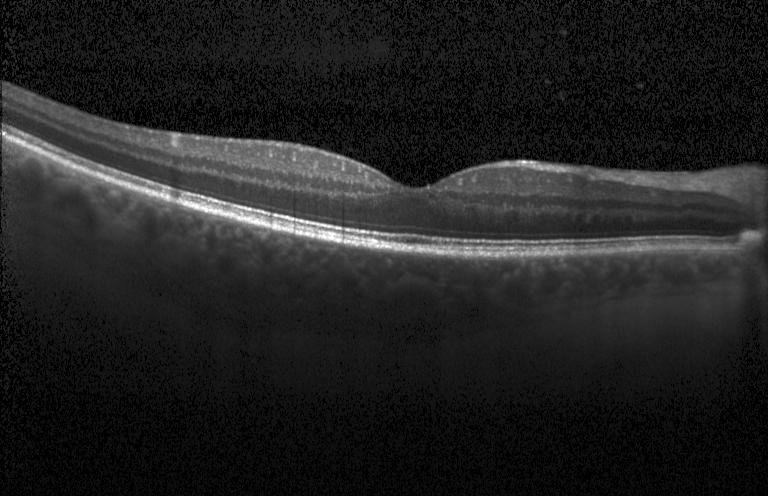
This B-scan demonstrates no choroidal neovascularization, diabetic macular edema, or drusen.